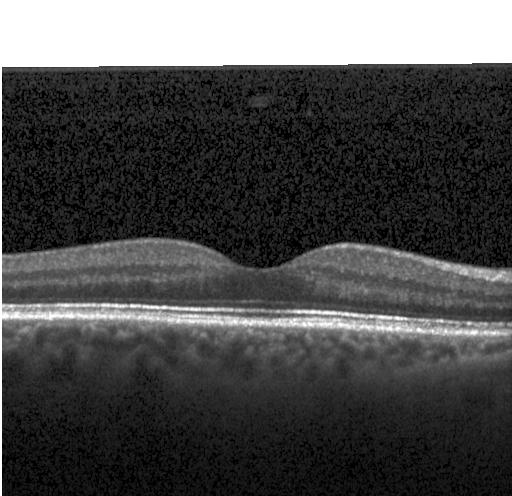

Heidelberg Spectralis OCT system, OCT line scan
The scan shows no evidence of choroidal neovascularization, diabetic macular edema, or drusen.